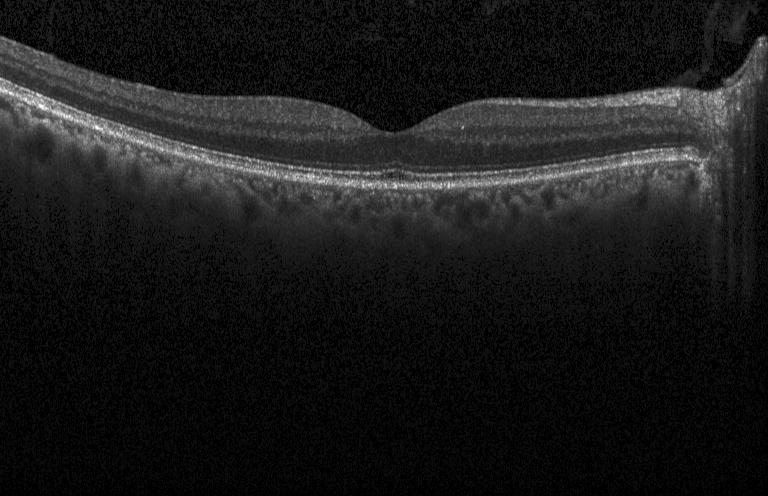 Finding: no evidence of choroidal neovascularization, diabetic macular edema, or drusen.